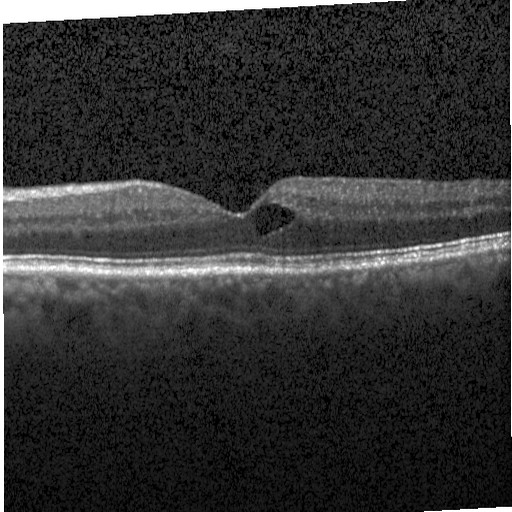

OCT scan showing diabetic macular edema.